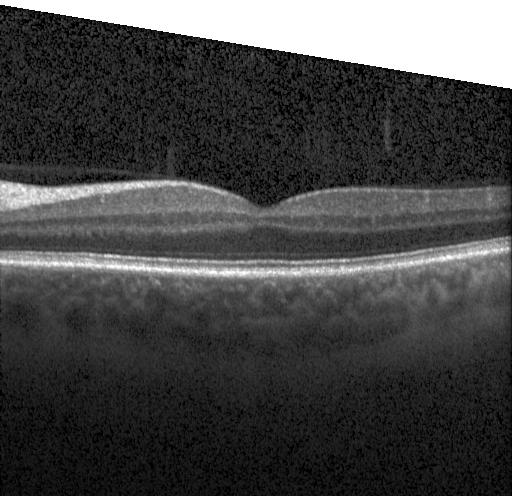

Finding: no CNV, DME, or drusen.